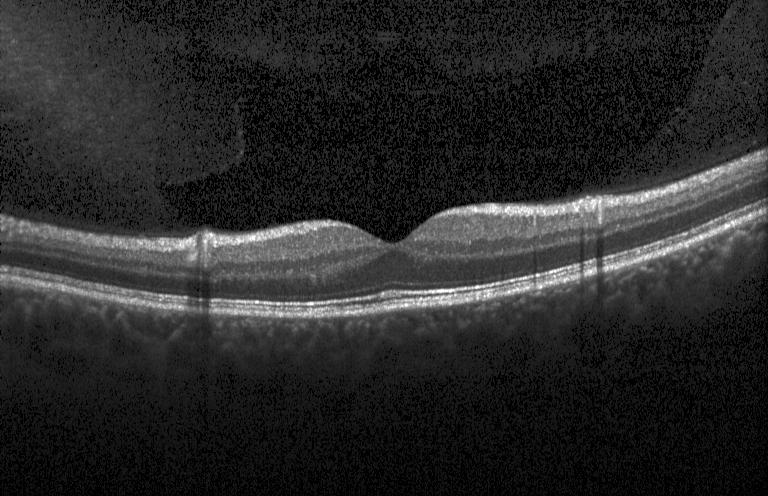 Horizontal scan through the fovea; OCT line scan — Diagnosis: neither choroidal neovascularization, diabetic macular edema, nor drusen.